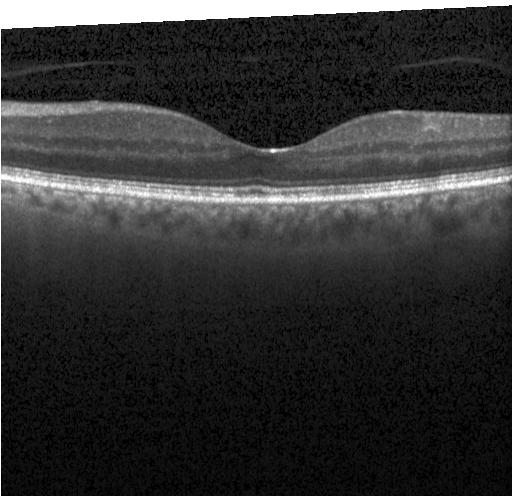

Fovea-centered · retinal OCT B-scan · SD-OCT · instrument: Heidelberg Spectralis — Finding: neither CNV, DME, nor drusen.